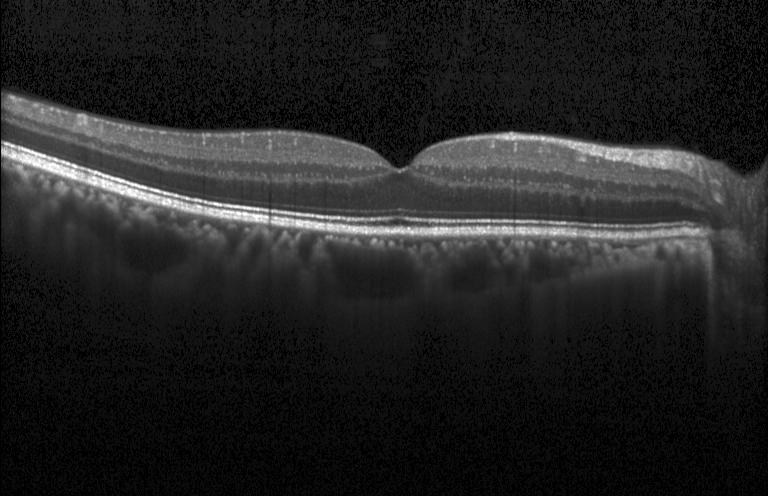
Heidelberg Spectralis, OCT B-scan — Macular OCT: no CNV, DME, or drusen.